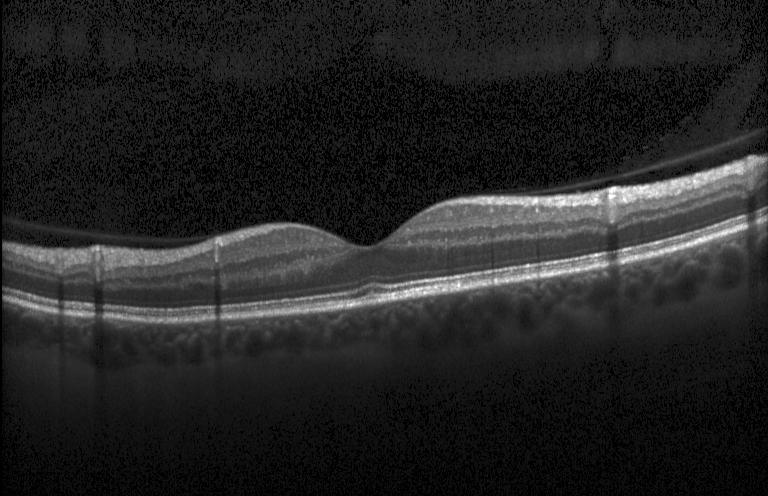 SD-OCT. Optical coherence tomography B-scan. Instrument: Heidelberg Spectralis
No choroidal neovascularization, diabetic macular edema, or drusen.